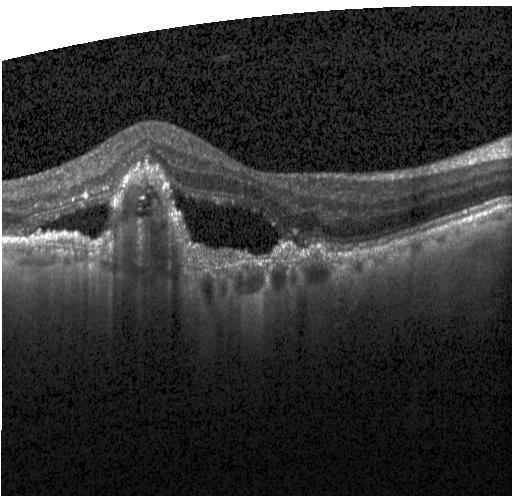

Retinal OCT B-scan. Diagnosis: choroidal neovascularization (CNV).